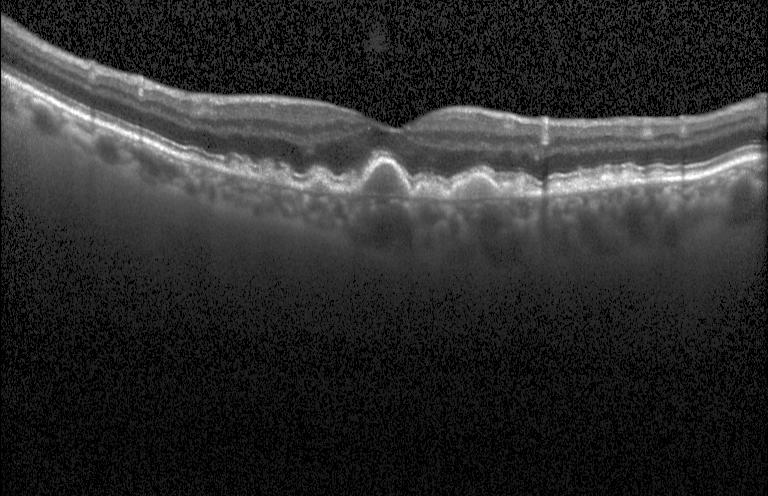

Finding: sub-RPE drusenoid deposits.